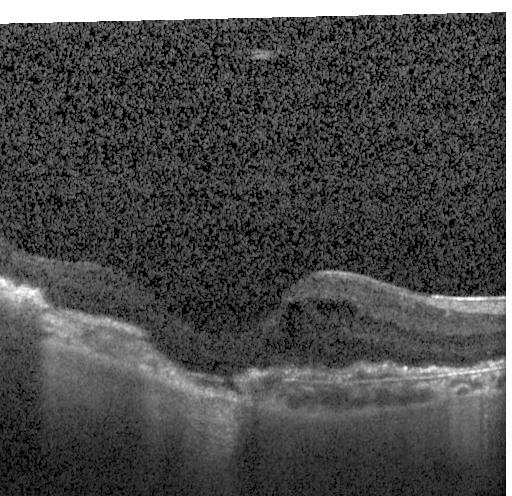
Instrument: Heidelberg Spectralis; optical coherence tomography scan; spectral-domain OCT; macular scan.
Diagnosis: choroidal neovascularization (CNV).